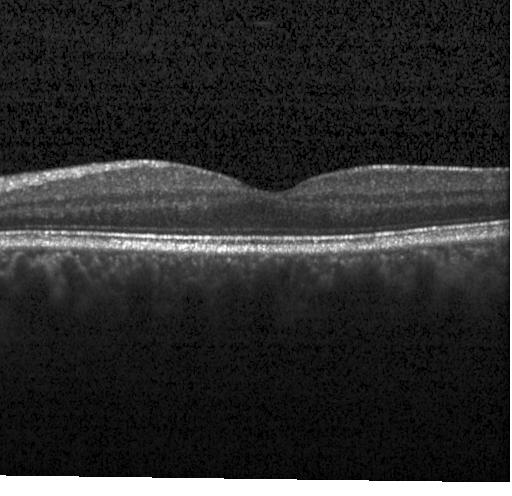
Optical coherence tomography B-scan.
Assessment: no choroidal neovascularization, diabetic macular edema, or drusen.